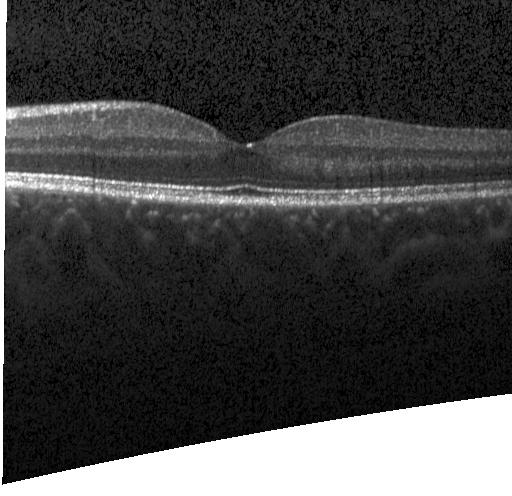

No evidence of choroidal neovascularization, diabetic macular edema, or drusen.